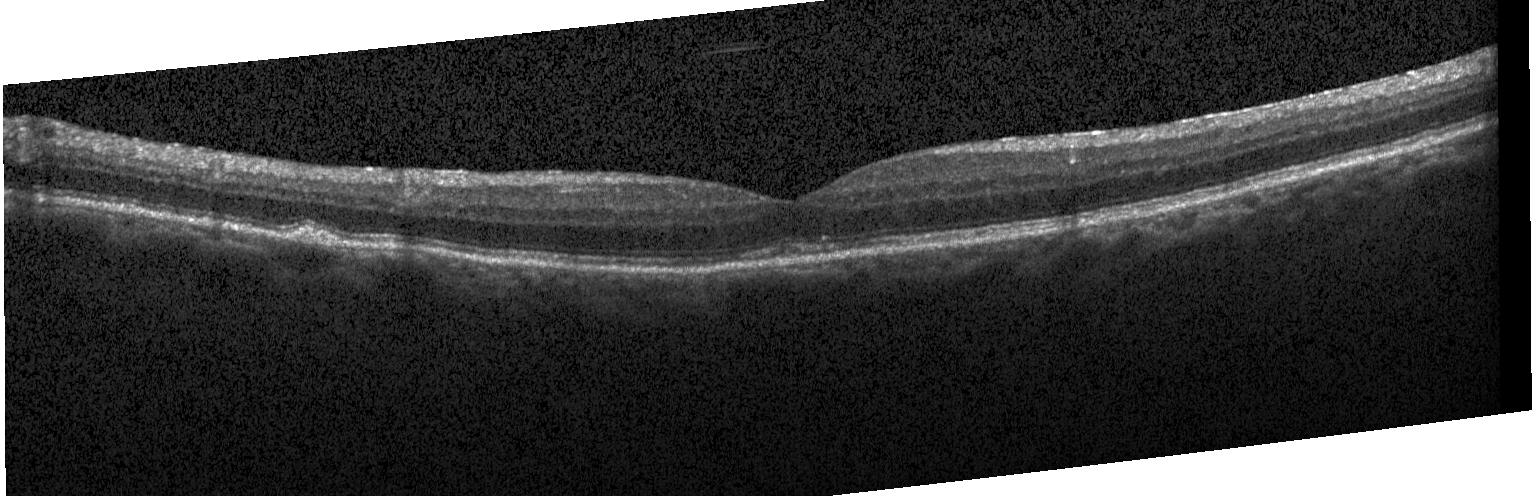
Diagnosis: sub-RPE drusenoid deposits.